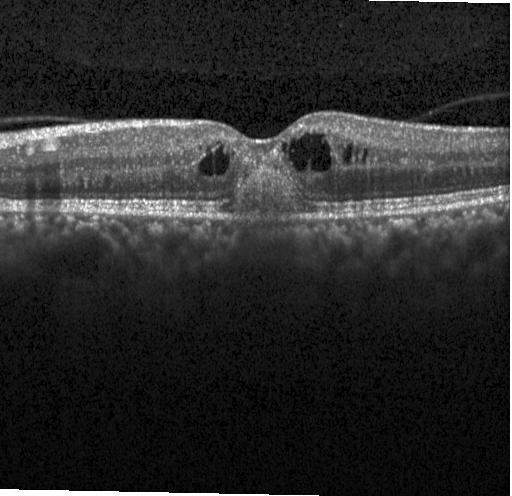
Finding: a choroidal neovascular membrane.